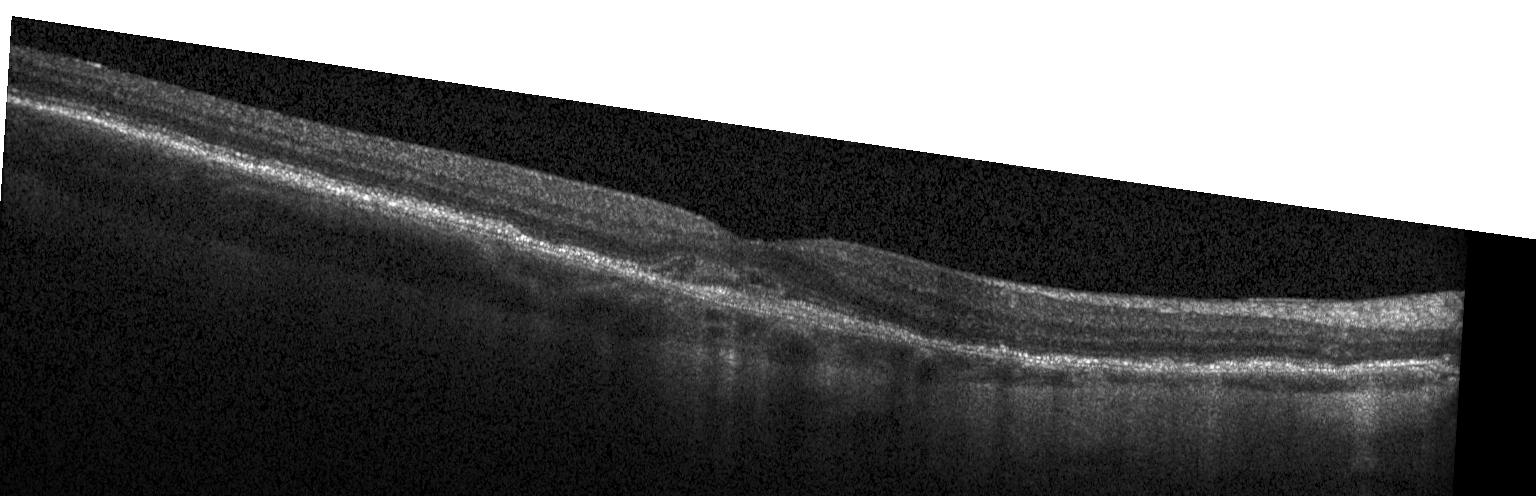
Retinal OCT B-scan
Impression: CNV.